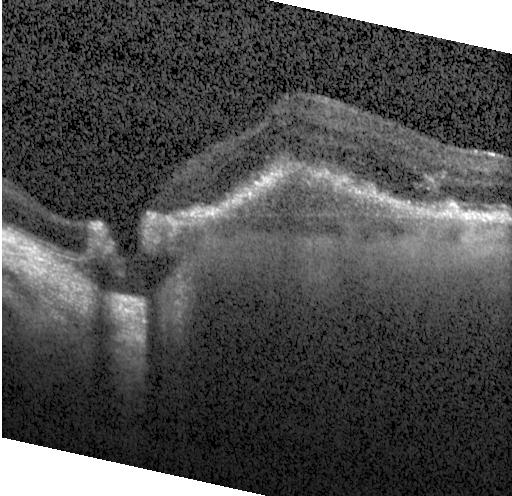 OCT B-scan, SD-OCT. Finding: a choroidal neovascular membrane.